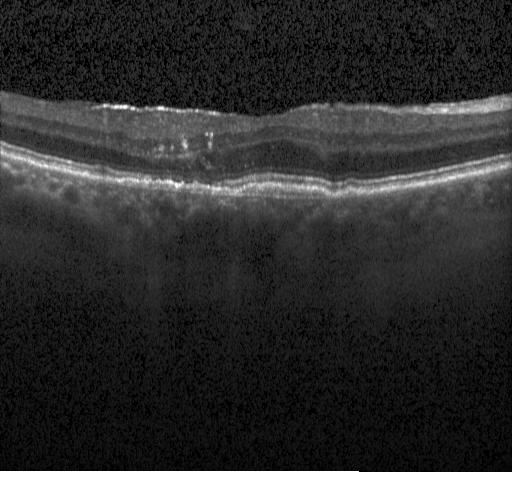
Spectral-domain OCT B-scan: choroidal neovascularization (CNV).